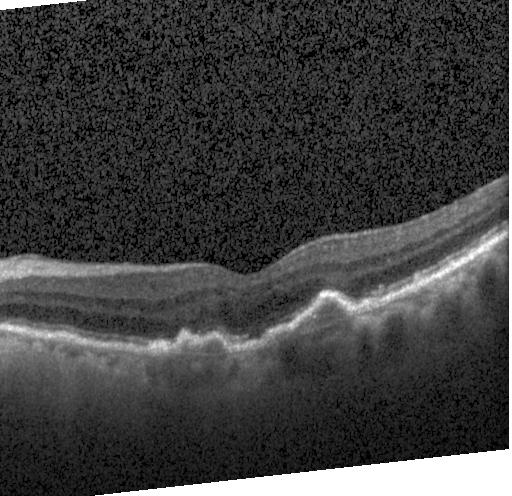 Finding: CNV.